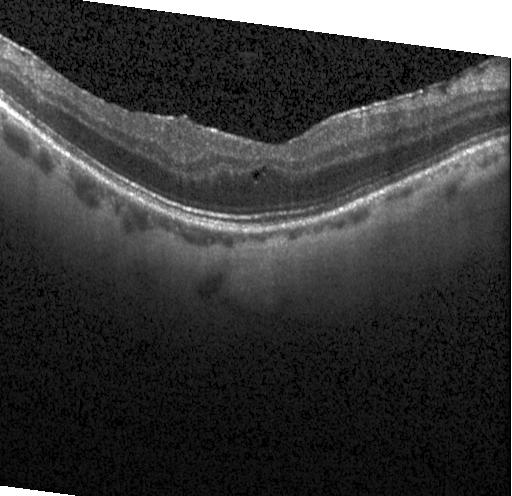
Dx: diabetic macular edema (DME).